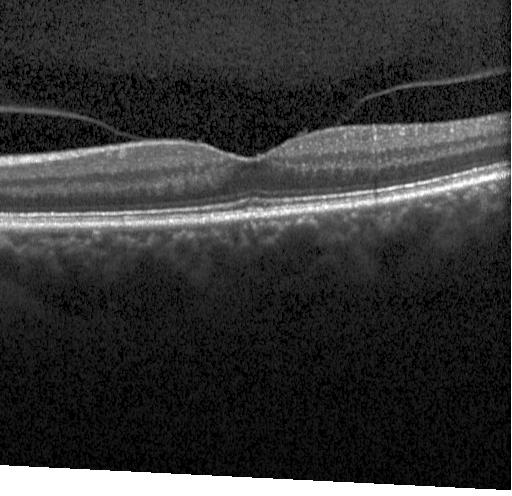 This B-scan demonstrates no CNV, DME, or drusen.